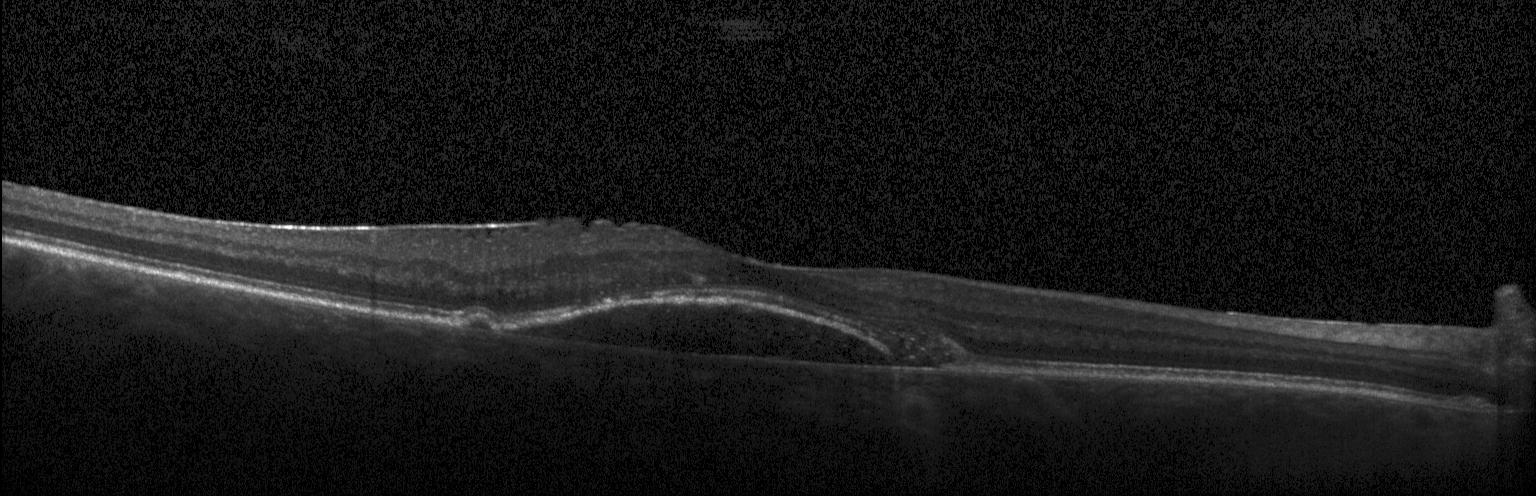

This B-scan demonstrates a choroidal neovascular membrane.